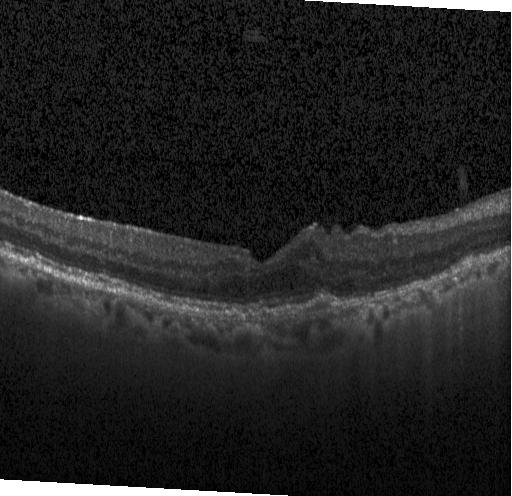 The scan shows a choroidal neovascular membrane.